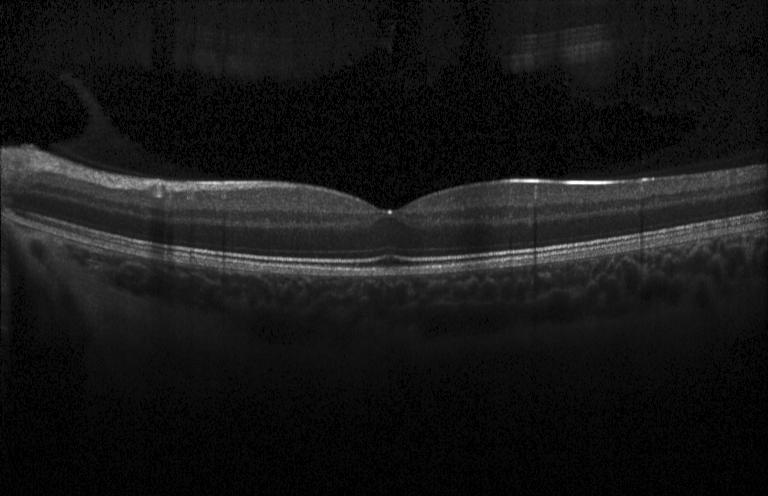 Through the macula. Retinal OCT cross-section
Diagnosis: no evidence of choroidal neovascularization, diabetic macular edema, or drusen.